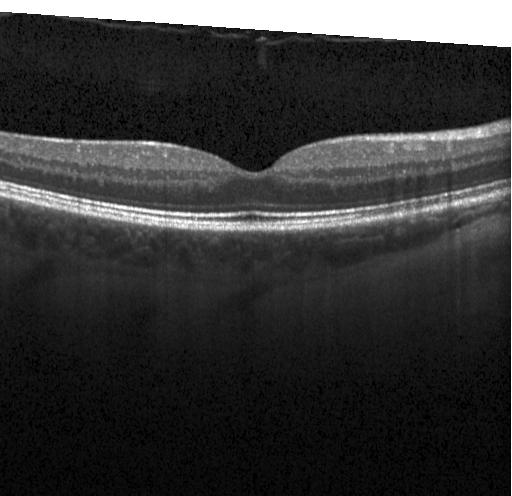

Impression: no CNV, no DME, and no drusen.